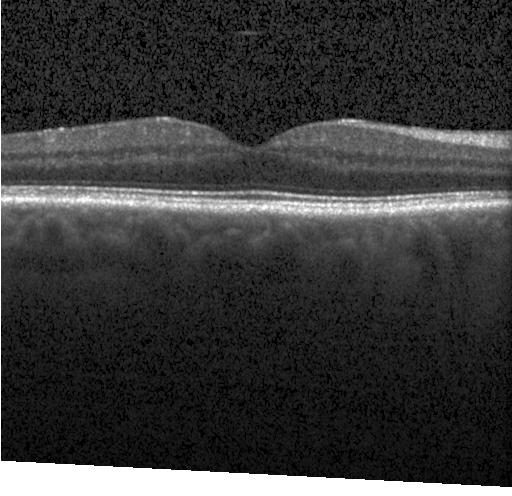 Macular OCT: no choroidal neovascularization, no diabetic macular edema, and no drusen.